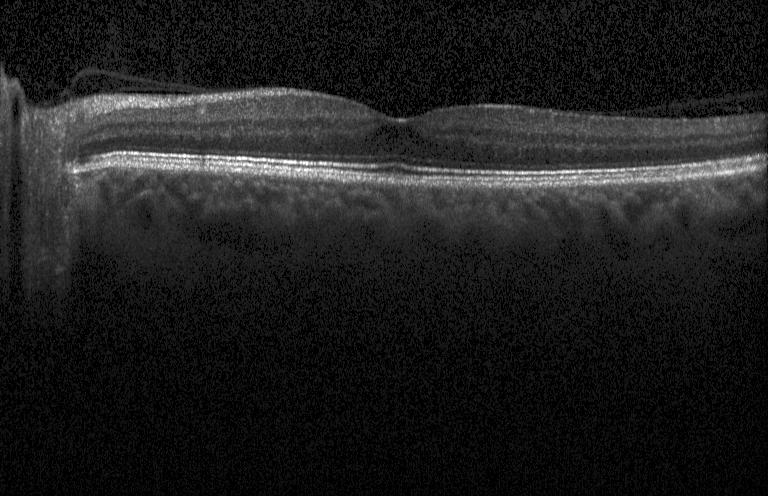
Macular OCT: neither choroidal neovascularization, diabetic macular edema, nor drusen.